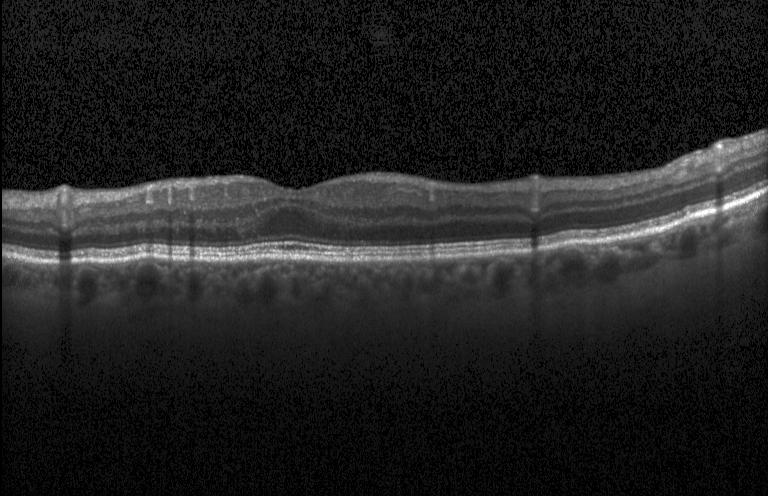 Acquired on a Heidelberg Spectralis, spectral-domain optical coherence tomography, retinal OCT cross-section. OCT finding: no choroidal neovascularization, diabetic macular edema, or drusen.